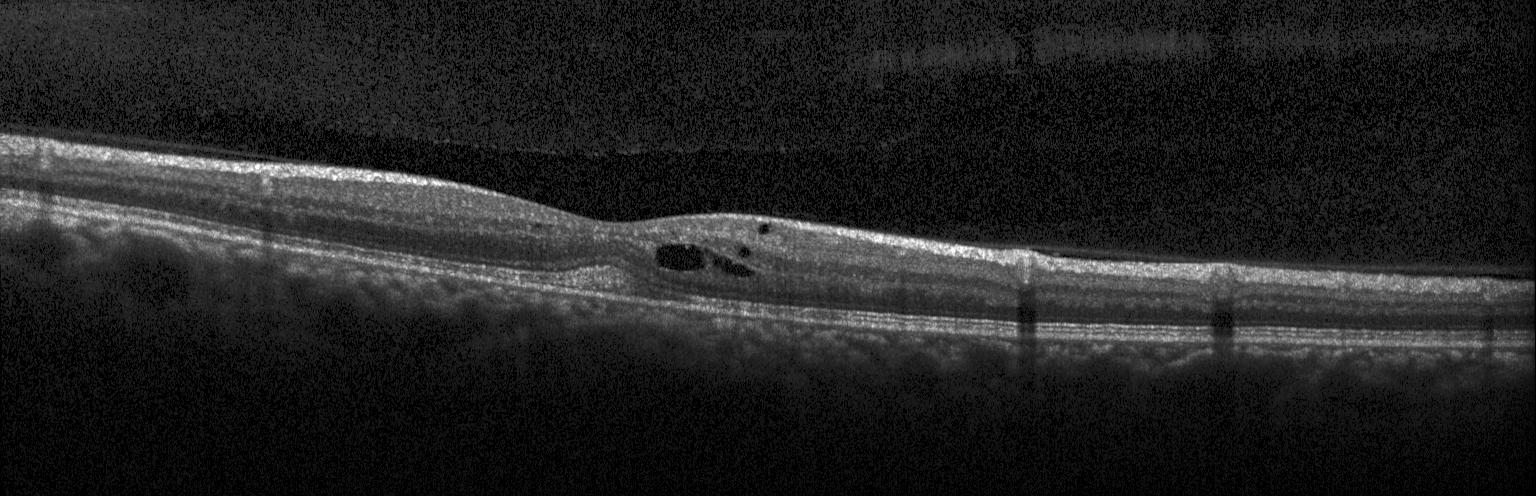 OCT B-scan. Finding: CNV.